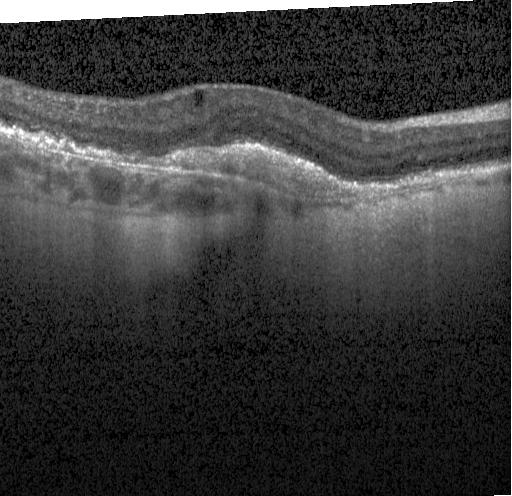

Optical coherence tomography scan
OCT finding: a choroidal neovascular membrane.